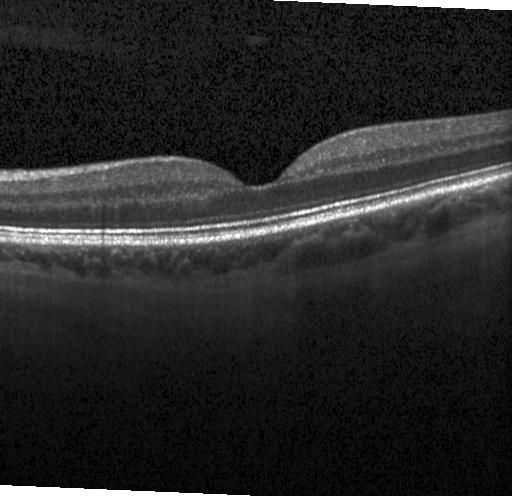 OCT finding: no evidence of choroidal neovascularization, diabetic macular edema, or drusen.